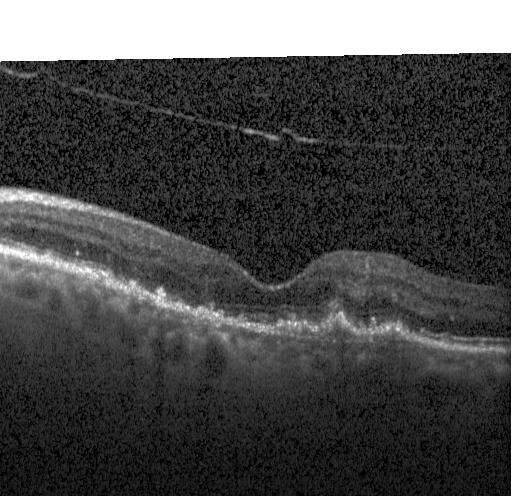
OCT line scan
Impression: choroidal neovascularization.